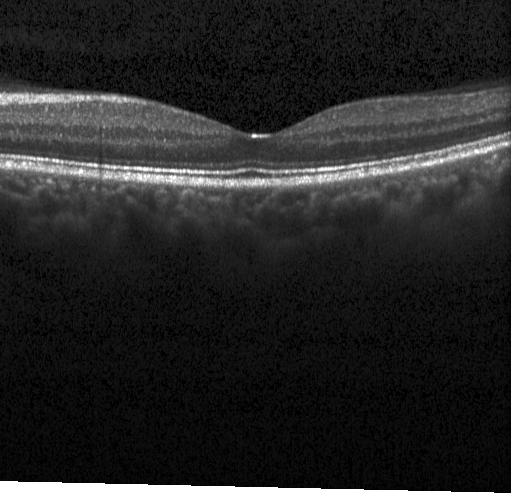
Fovea-centered. OCT line scan. Heidelberg Spectralis OCT system — Impression: neither choroidal neovascularization, diabetic macular edema, nor drusen.